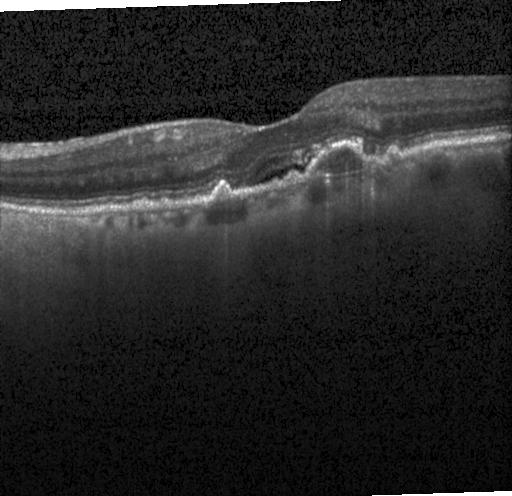 Retinal OCT cross-section, instrument: Heidelberg Spectralis.
Diagnosis: a choroidal neovascular membrane.